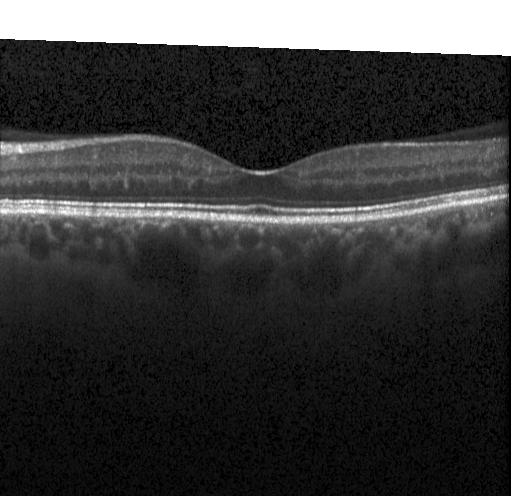 This B-scan demonstrates no evidence of CNV, DME, or drusen.